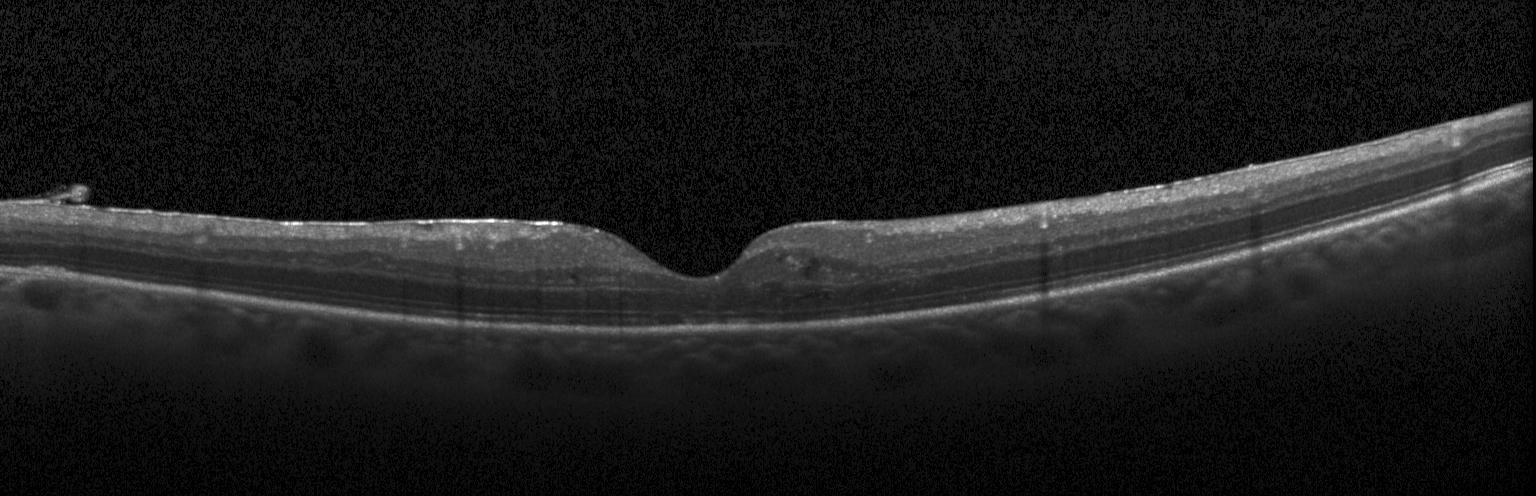 SD-OCT. Retinal OCT B-scan. Assessment: diabetic macular edema (DME).